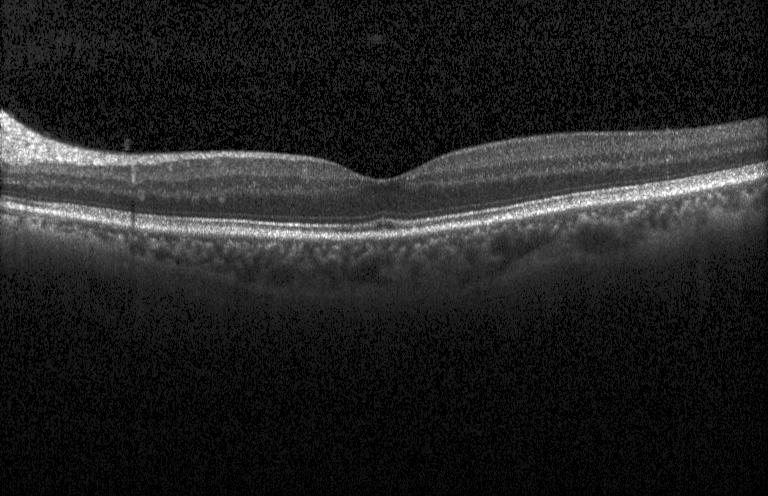
Heidelberg Spectralis · macular scan · SD-OCT · retinal OCT B-scan
Impression: no CNV, no DME, and no drusen.